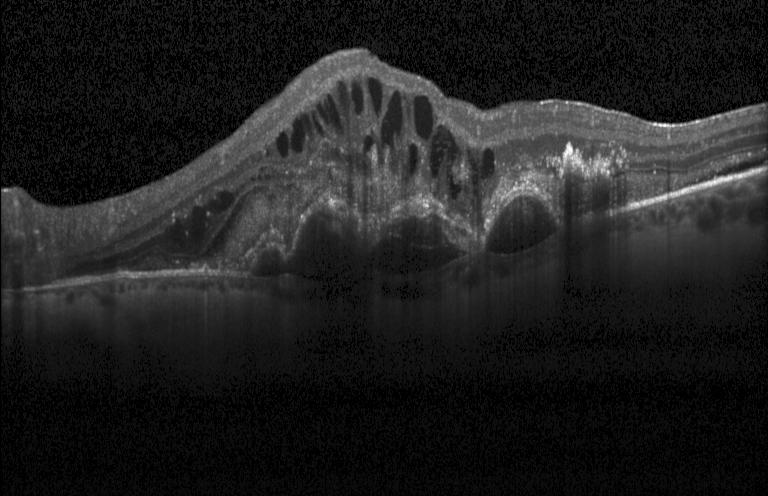
Dx: a choroidal neovascular membrane.